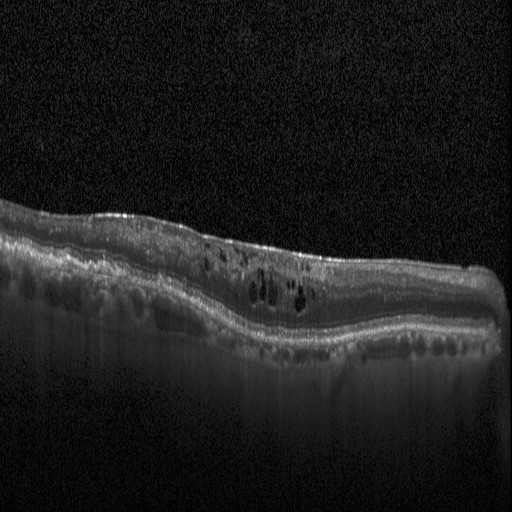 SD-OCT, fovea-centered, retinal OCT cross-section
Impression: diabetic macular edema.